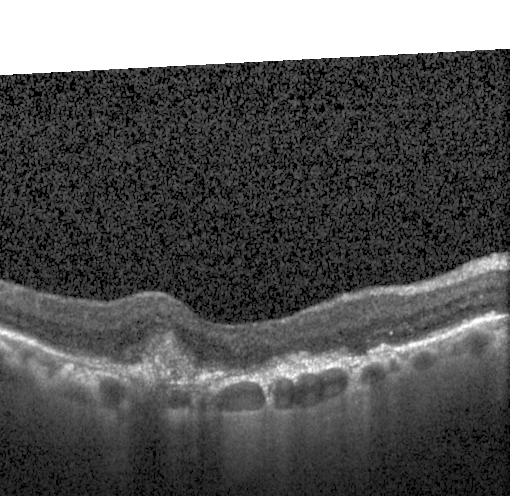
OCT B-scan showing choroidal neovascularization (CNV).